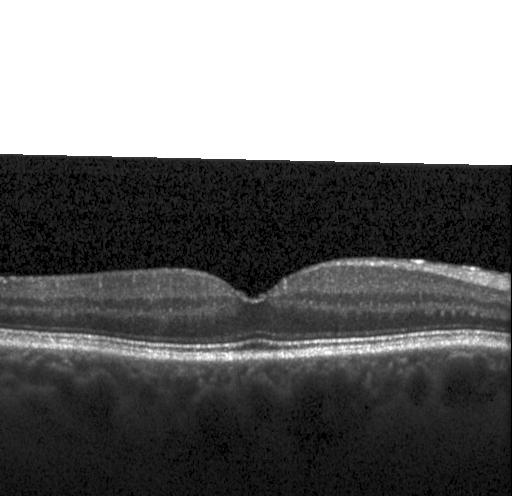 Spectral-domain optical coherence tomography, retinal OCT cross-section.
Diagnosis: neither CNV, DME, nor drusen.